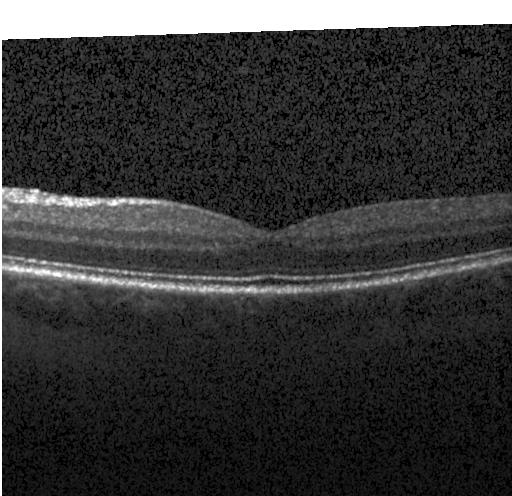

SD-OCT; Heidelberg Spectralis OCT system; optical coherence tomography scan. Diagnosis: no evidence of choroidal neovascularization, diabetic macular edema, or drusen.